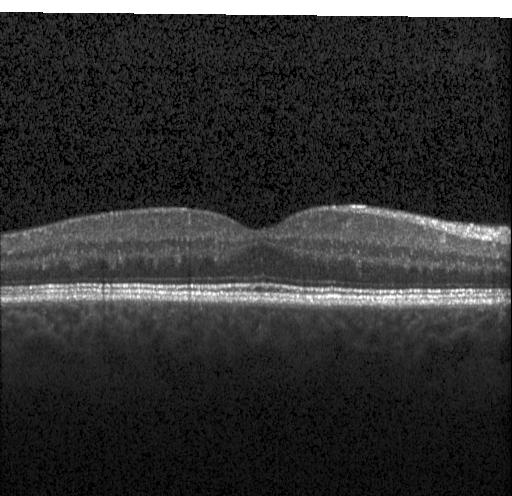

Acquired on a Heidelberg Spectralis; optical coherence tomography B-scan; macular scan
Dx: no choroidal neovascularization, diabetic macular edema, or drusen.